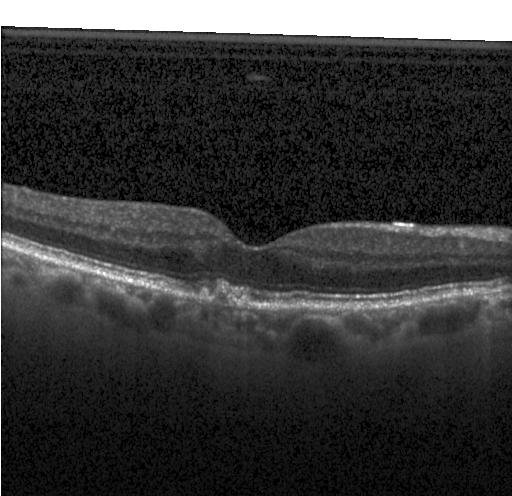
Diagnosis: multiple drusen.